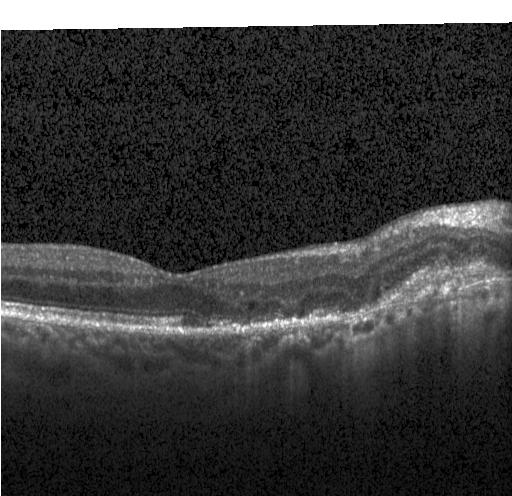
OCT line scan · spectral-domain optical coherence tomography · horizontal scan through the fovea · Heidelberg Spectralis.
Diagnosis: choroidal neovascularization.